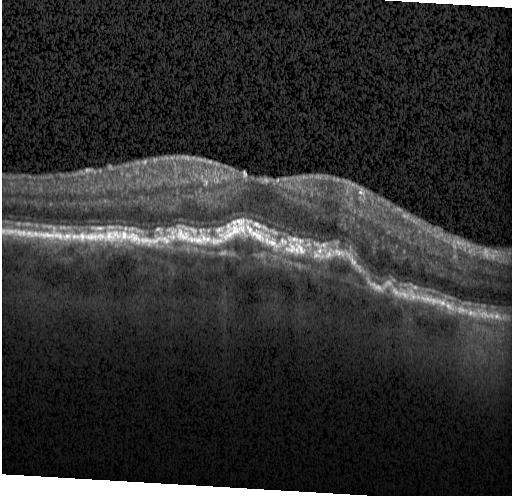
Optical coherence tomography B-scan · instrument: Heidelberg Spectralis · centered on the fovea
Macular OCT: a choroidal neovascular membrane.